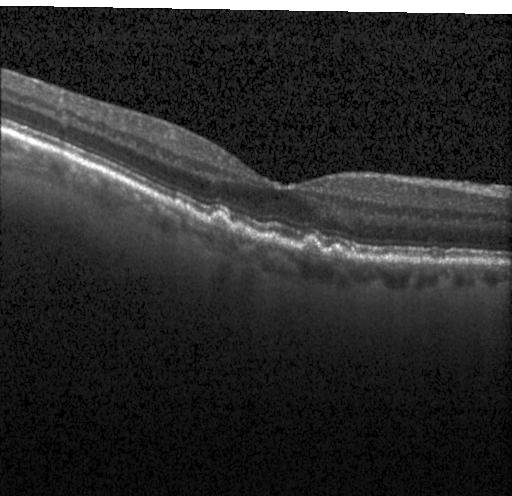

Spectral-domain optical coherence tomography. OCT B-scan. Instrument: Heidelberg Spectralis. The scan shows multiple drusen.